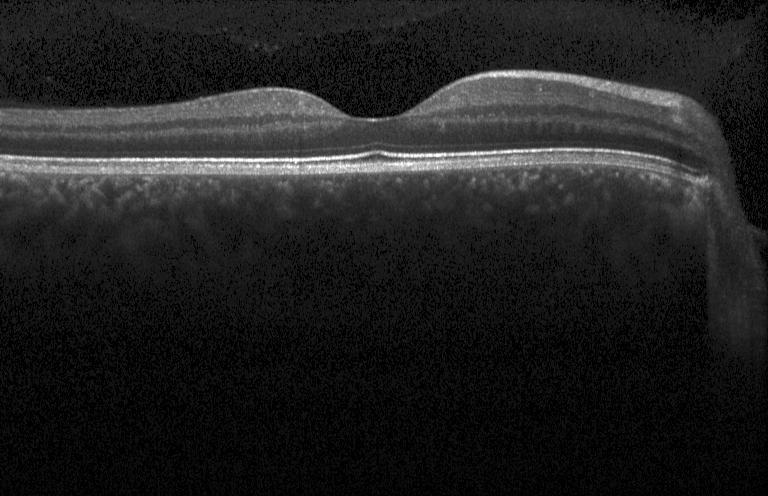 Instrument: Heidelberg Spectralis; optical coherence tomography B-scan.
Impression: no choroidal neovascularization, diabetic macular edema, or drusen.